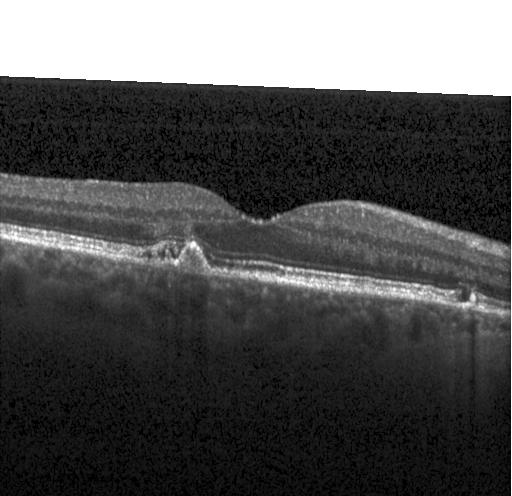
This B-scan demonstrates CNV.